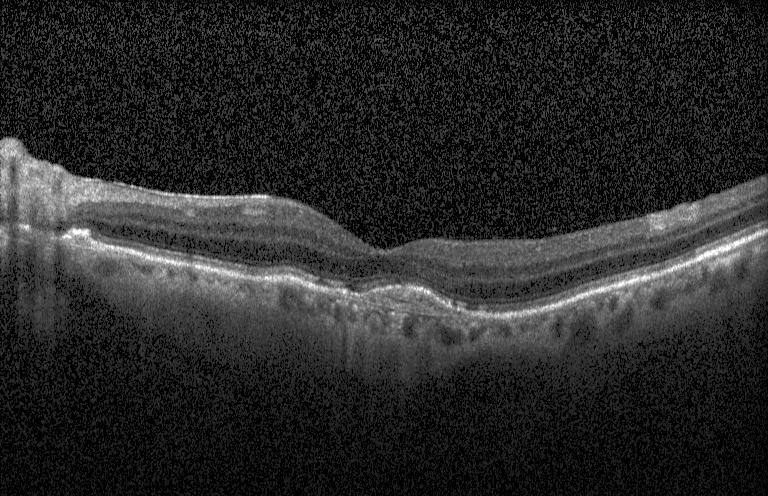
Optical coherence tomography B-scan · Heidelberg Spectralis · spectral-domain optical coherence tomography · centered on the fovea. Impression: choroidal neovascularization (CNV).